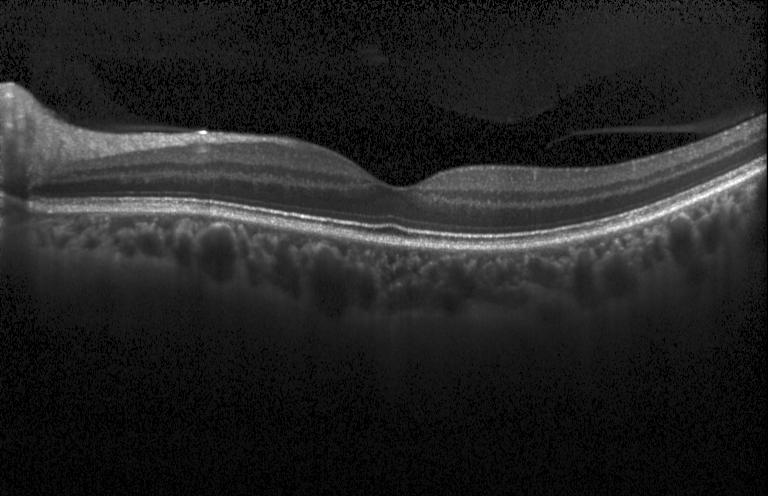
Macular OCT: no evidence of choroidal neovascularization, diabetic macular edema, or drusen.